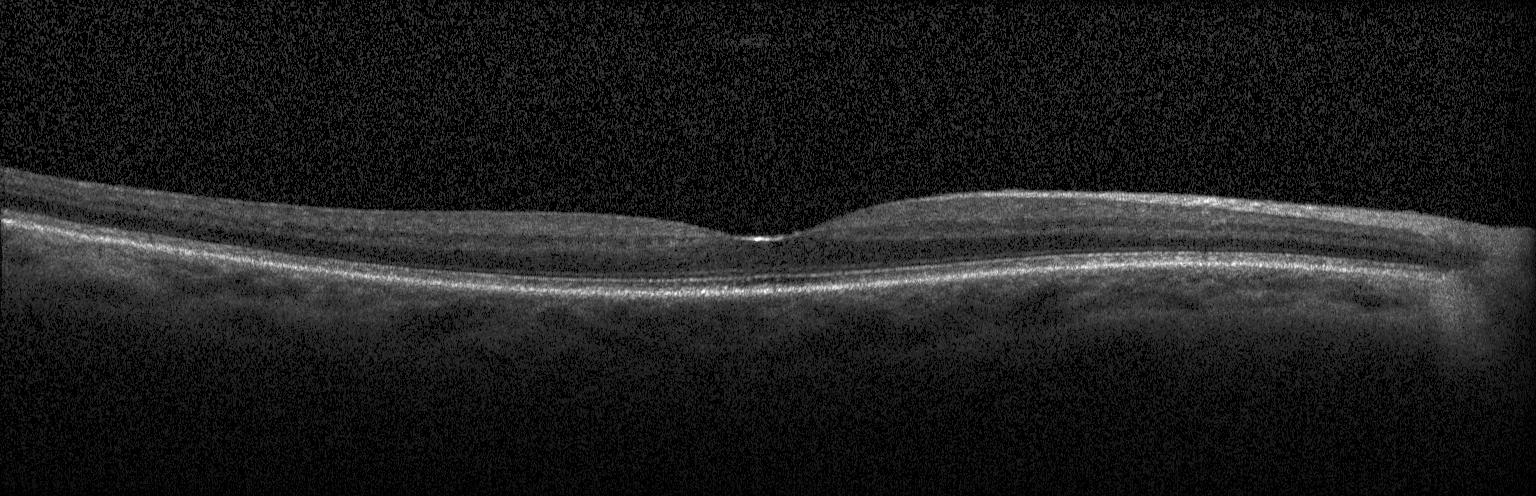
Optical coherence tomography B-scan
Diagnosis: neither choroidal neovascularization, diabetic macular edema, nor drusen.